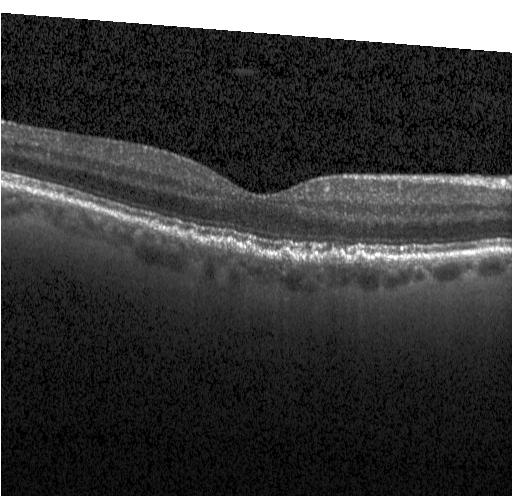

Dx: drusen.